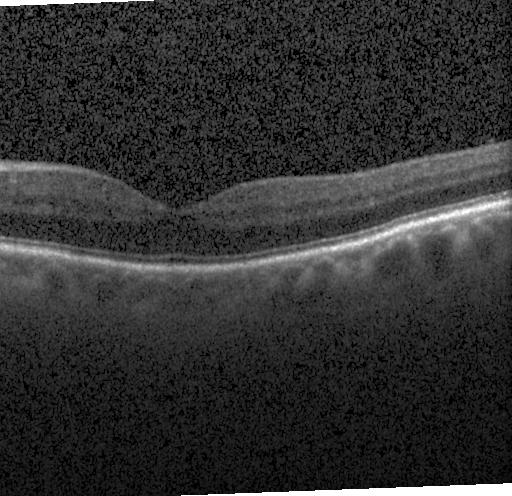

Acquired on a Heidelberg Spectralis, spectral-domain OCT, OCT B-scan, fovea-centered.
Diagnosis: neither choroidal neovascularization, diabetic macular edema, nor drusen.